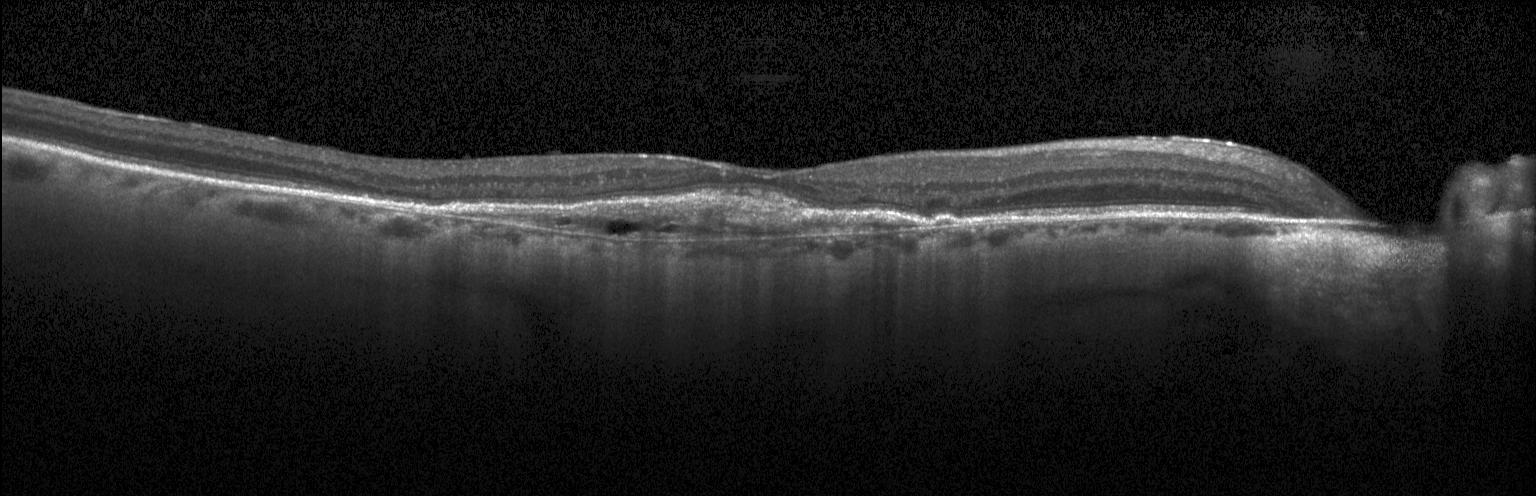 Spectral-domain optical coherence tomography. Optical coherence tomography B-scan. Instrument: Heidelberg Spectralis. Fovea-centered
Diagnosis: a choroidal neovascular membrane.